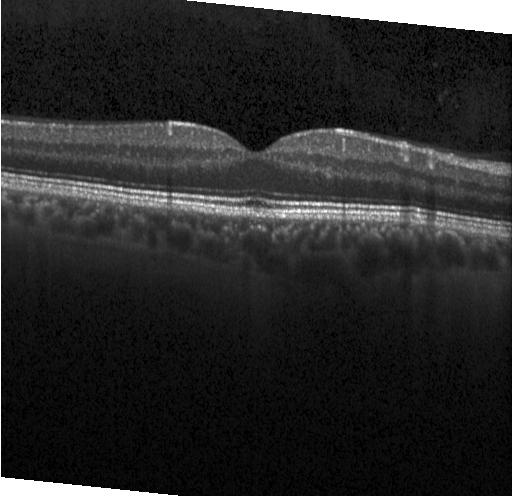

Spectral-domain OCT, optical coherence tomography scan
Macular OCT: no choroidal neovascularization, no diabetic macular edema, and no drusen.